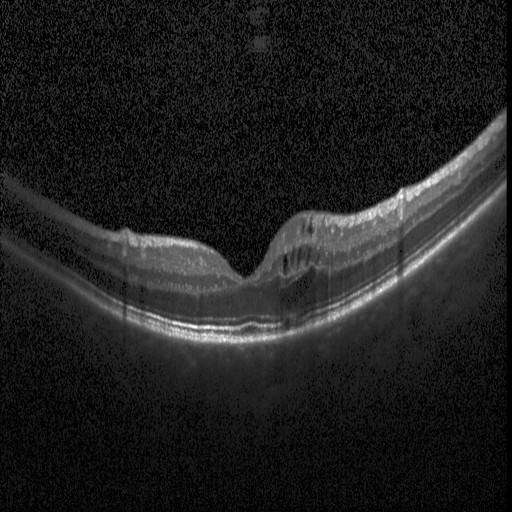 SD-OCT · retinal OCT B-scan.
Dx: diabetic macular edema.